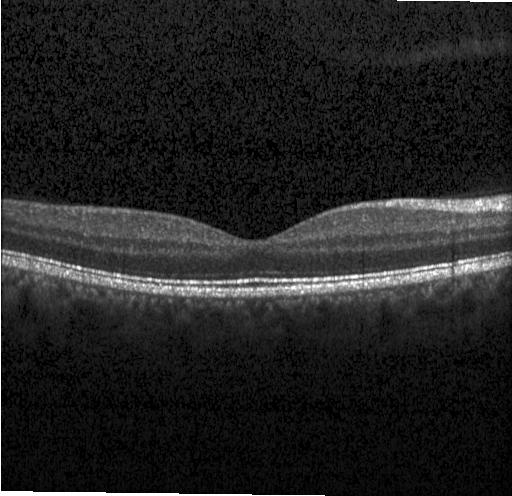

Retinal OCT cross-section · centered on the fovea. Macular OCT: neither choroidal neovascularization, diabetic macular edema, nor drusen.